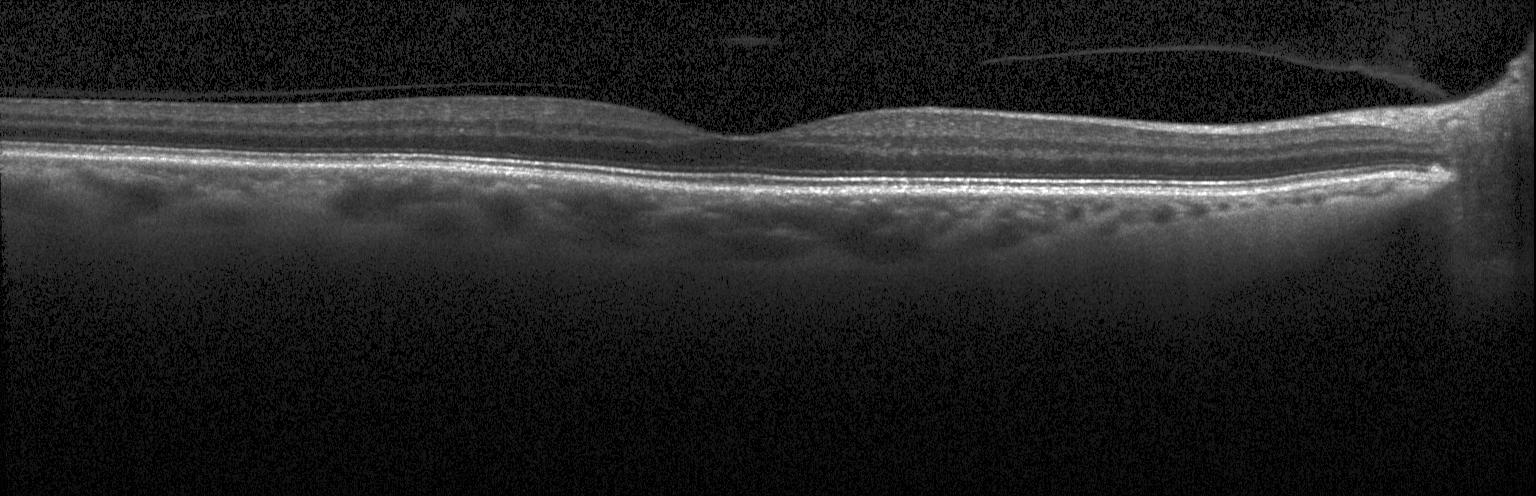
SD-OCT; horizontal scan through the fovea; retinal OCT cross-section — Impression: no evidence of choroidal neovascularization, diabetic macular edema, or drusen.